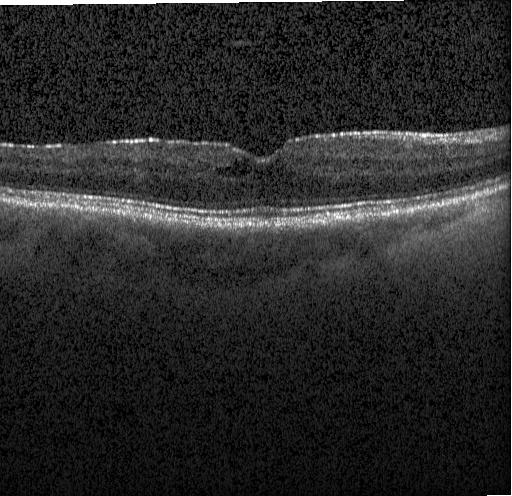

OCT finding: DME.